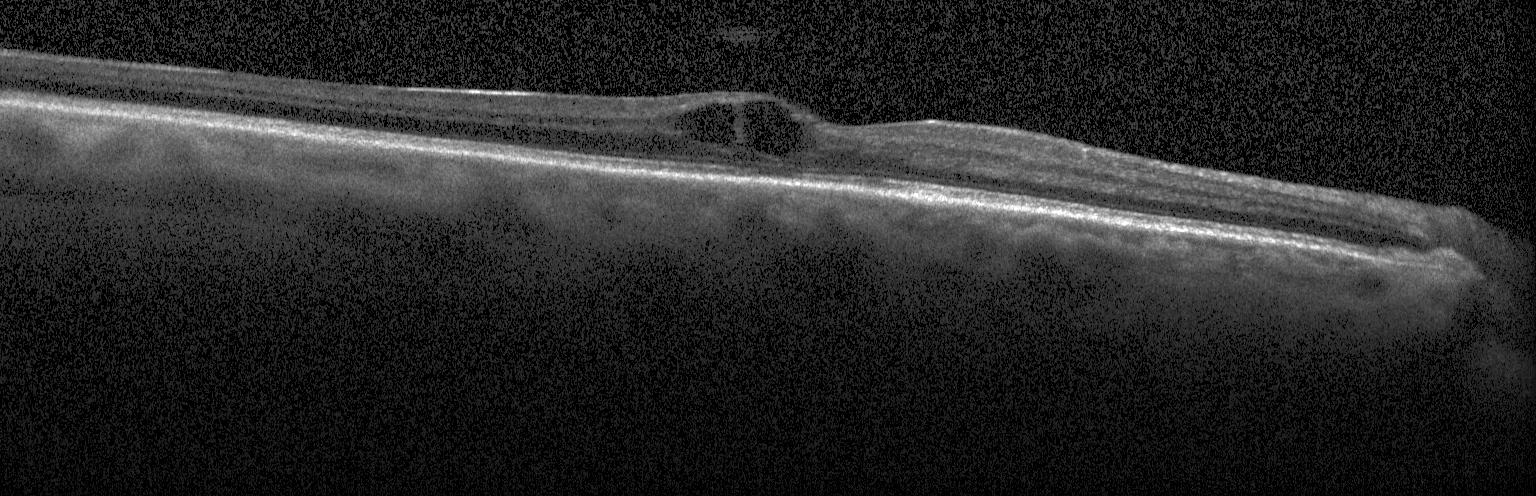 The scan shows DME.